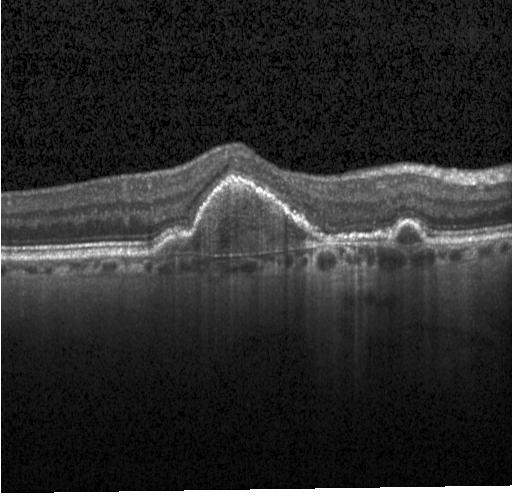
A choroidal neovascular membrane.